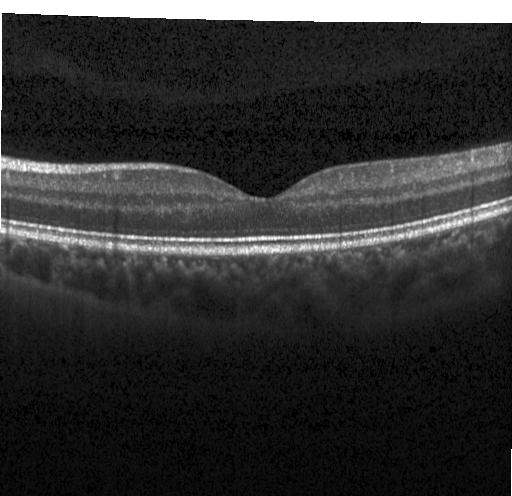
Optical coherence tomography scan · macular scan · SD-OCT · instrument: Heidelberg Spectralis — Impression: neither CNV, DME, nor drusen.